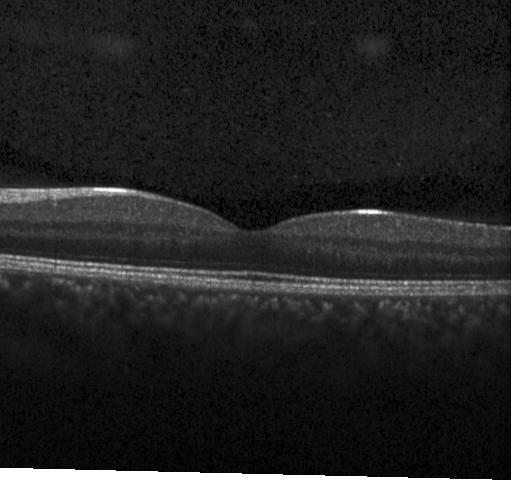
This B-scan demonstrates neither CNV, DME, nor drusen.